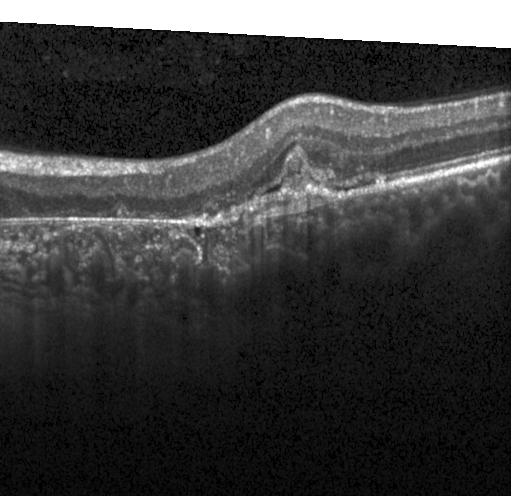
Spectral-domain OCT B-scan: choroidal neovascularization (CNV).